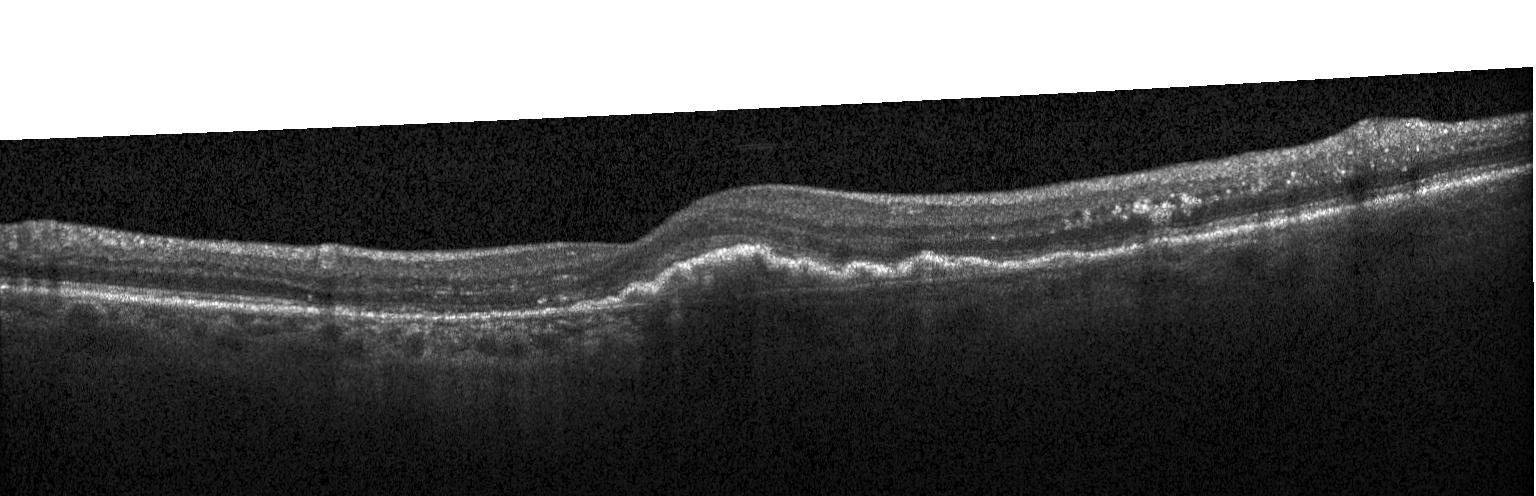 Spectral-domain optical coherence tomography; optical coherence tomography scan.
Impression: a choroidal neovascular membrane.